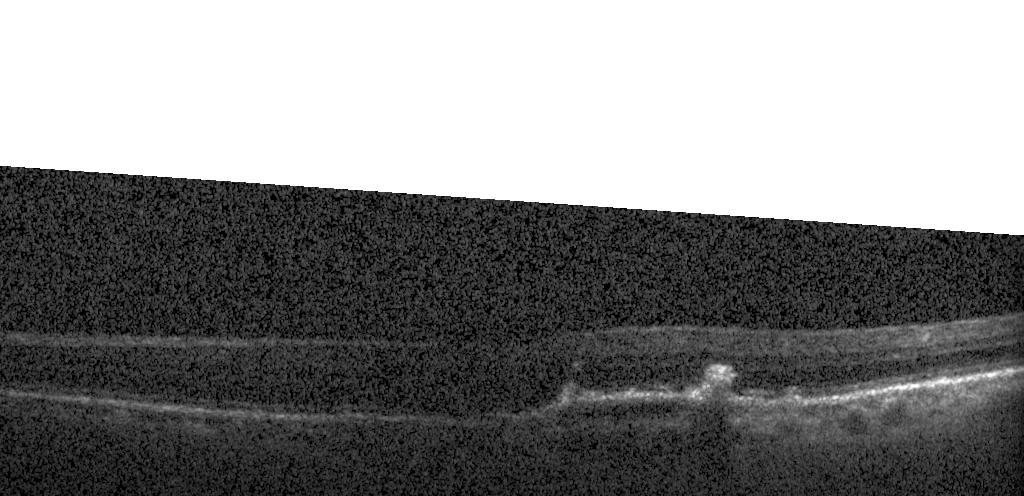 OCT line scan. Acquired on a Heidelberg Spectralis. Spectral-domain optical coherence tomography. Macular scan — OCT finding: choroidal neovascularization (CNV).